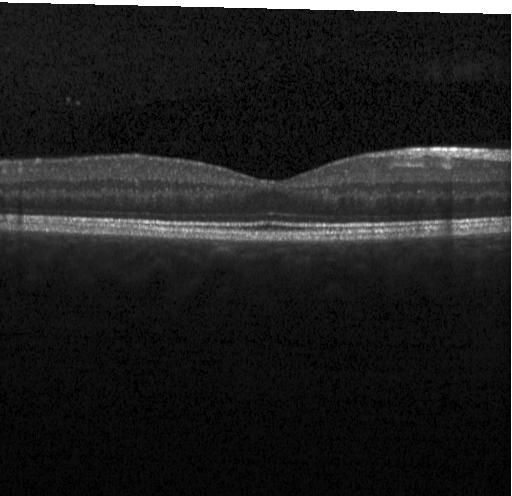
Optical coherence tomography B-scan
OCT finding: neither choroidal neovascularization, diabetic macular edema, nor drusen.